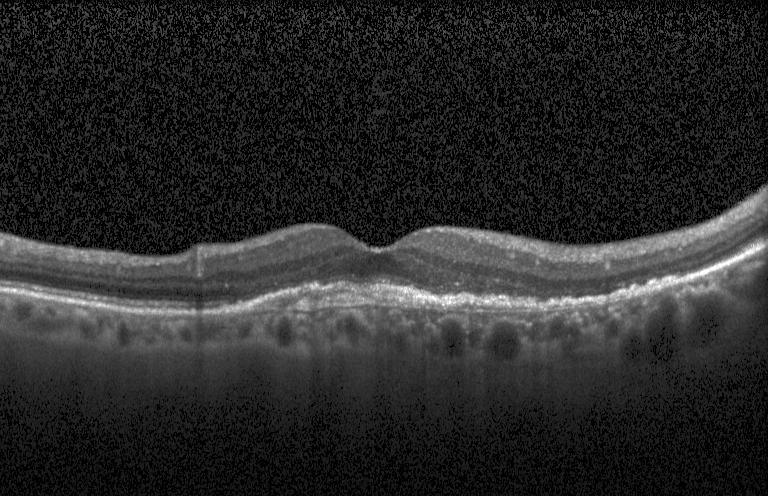
Finding: a choroidal neovascular membrane.